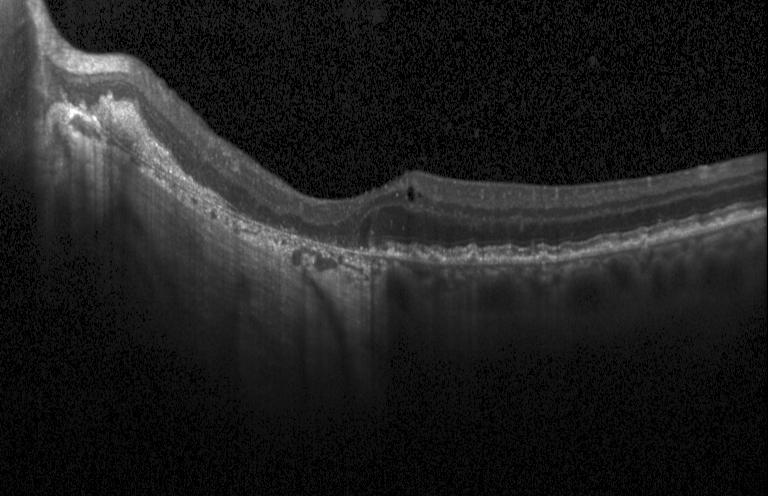 OCT B-scan. Diagnosis: a choroidal neovascular membrane.